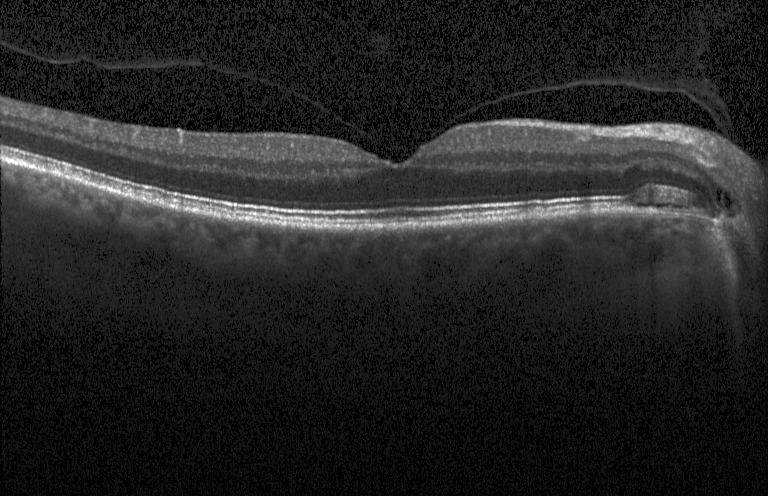

Horizontal scan through the fovea. Optical coherence tomography scan. Spectral-domain OCT. Instrument: Heidelberg Spectralis — This B-scan demonstrates no evidence of choroidal neovascularization, diabetic macular edema, or drusen.